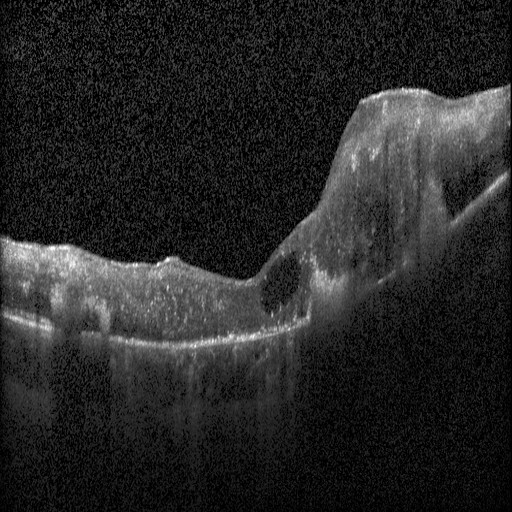
Retinal OCT cross-section · spectral-domain optical coherence tomography · centered on the fovea · acquired on a Heidelberg Spectralis. Diagnosis: diabetic macular edema (DME).